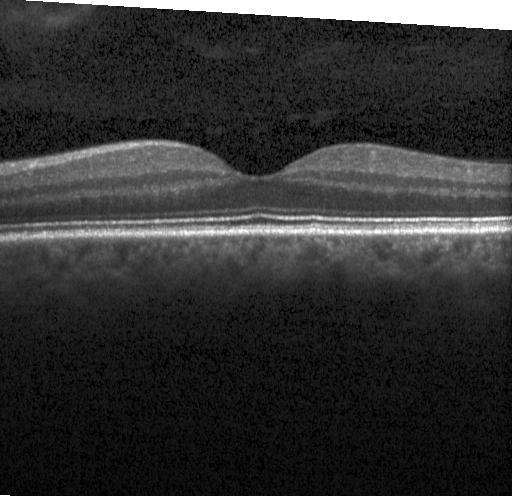

Horizontal scan through the fovea · spectral-domain optical coherence tomography · optical coherence tomography scan.
Finding: no evidence of choroidal neovascularization, diabetic macular edema, or drusen.